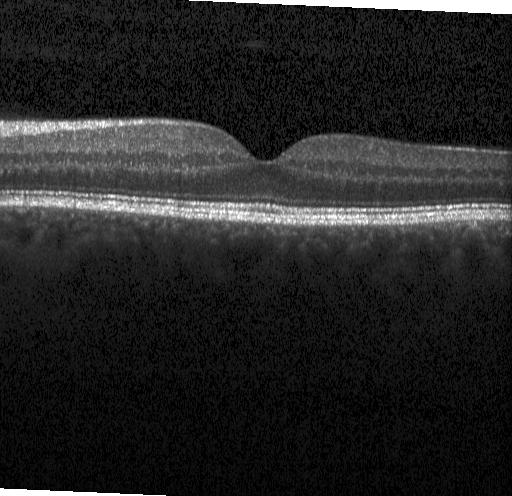 OCT scan showing no choroidal neovascularization, diabetic macular edema, or drusen.